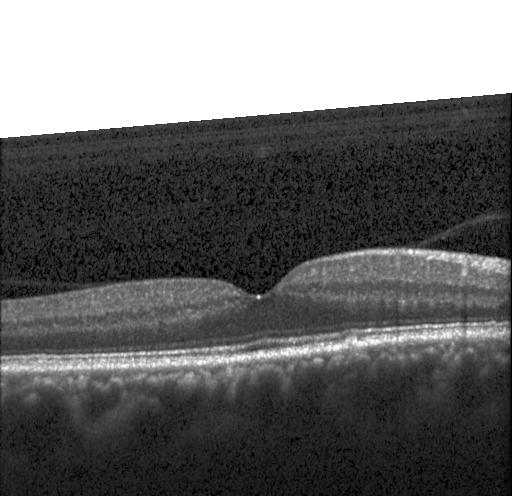

SD-OCT; OCT line scan; acquired on a Heidelberg Spectralis
Diagnosis: no CNV, DME, or drusen.